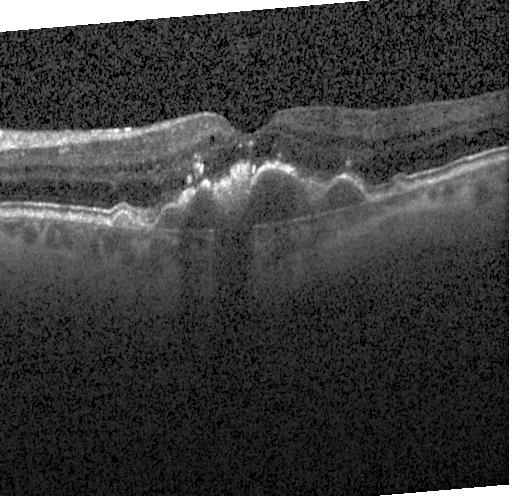

Dx: choroidal neovascularization (CNV).